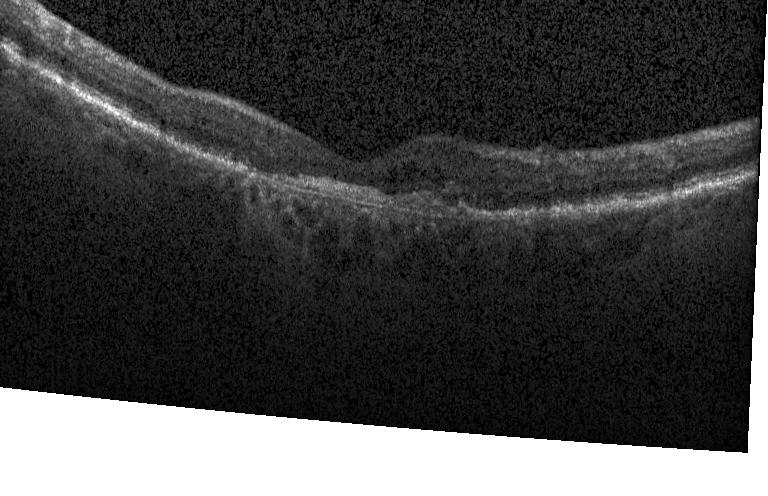

Acquired on a Heidelberg Spectralis · spectral-domain OCT · retinal OCT cross-section · through the macula. OCT finding: a choroidal neovascular membrane.